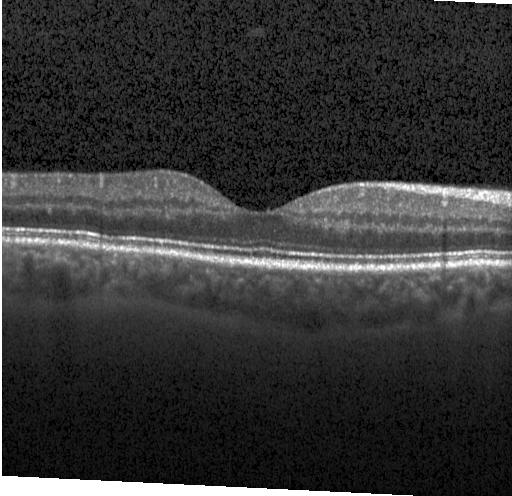 OCT line scan. Diagnosis: no CNV, no DME, and no drusen.